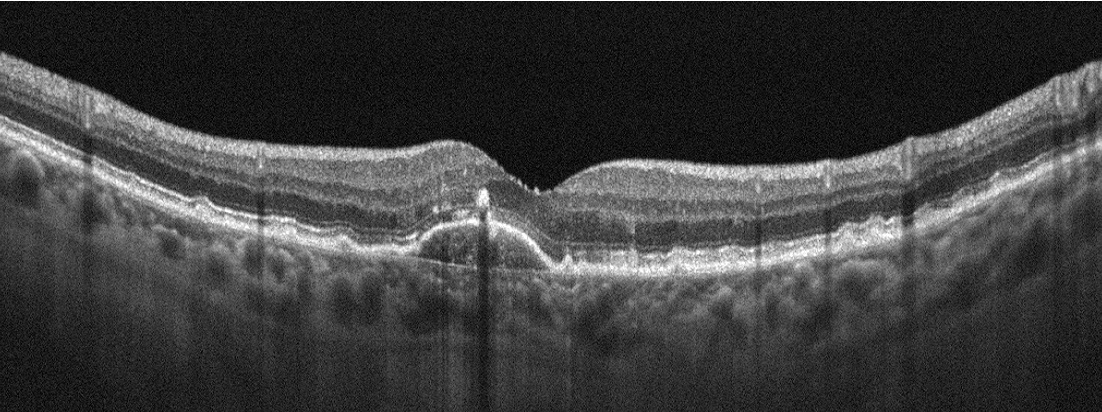

Assessment: AMD.